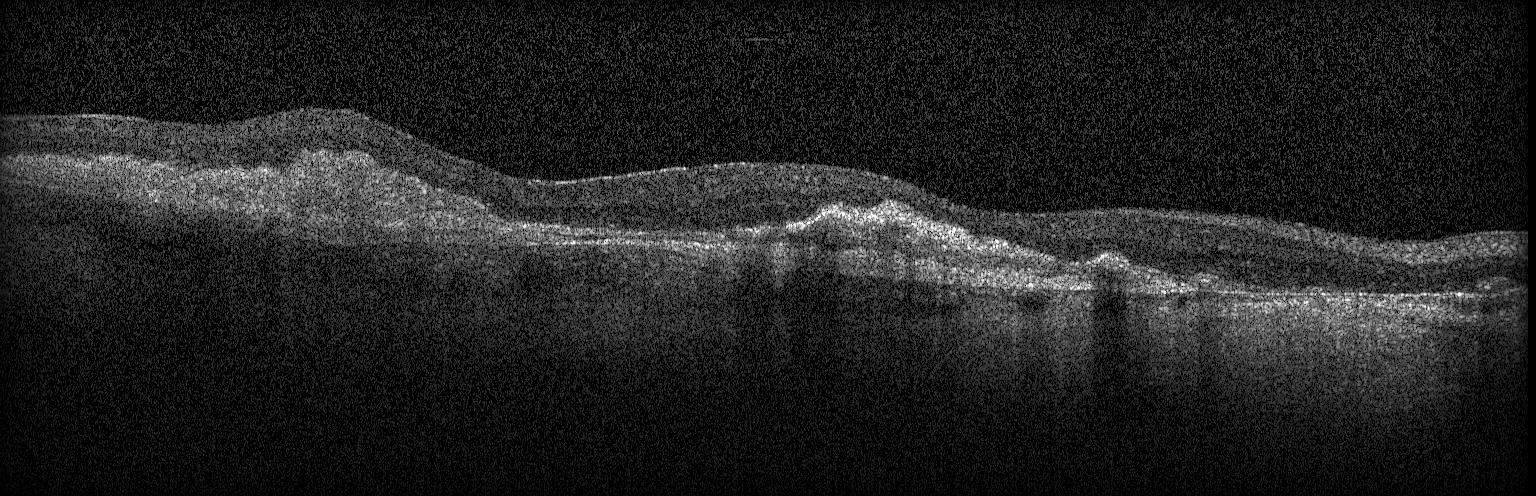 Optical coherence tomography B-scan · acquired on a Heidelberg Spectralis. Assessment: CNV.